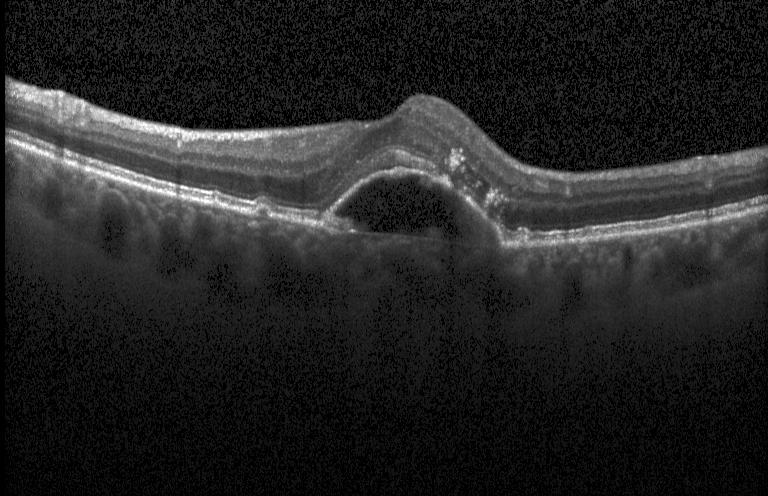
Spectral-domain OCT; retinal OCT B-scan; Heidelberg Spectralis; through the macula
This B-scan demonstrates a choroidal neovascular membrane.